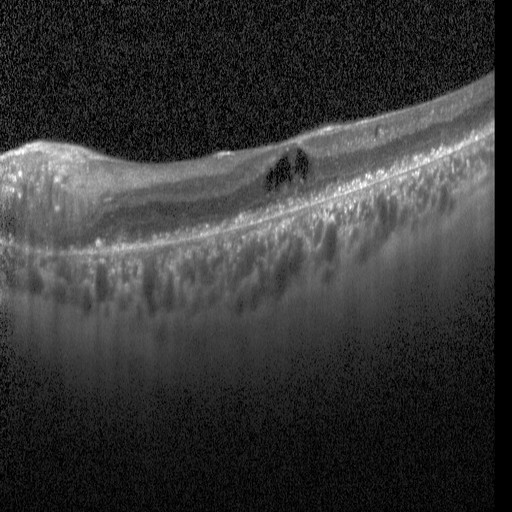

Dx: diabetic macular edema (DME).